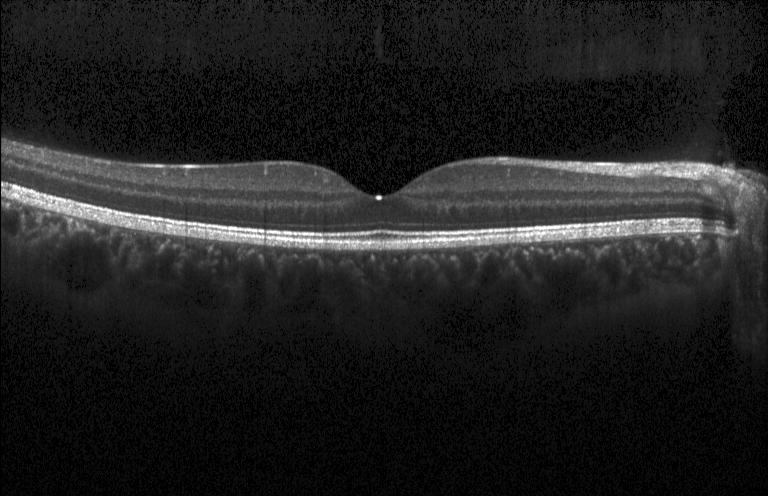 Macular OCT: no choroidal neovascularization, diabetic macular edema, or drusen.